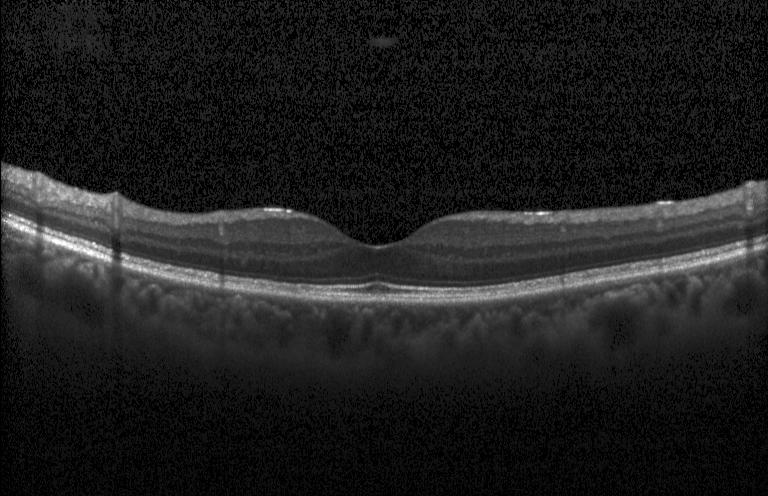 OCT B-scan · macular scan — Diagnosis: no choroidal neovascularization, diabetic macular edema, or drusen.